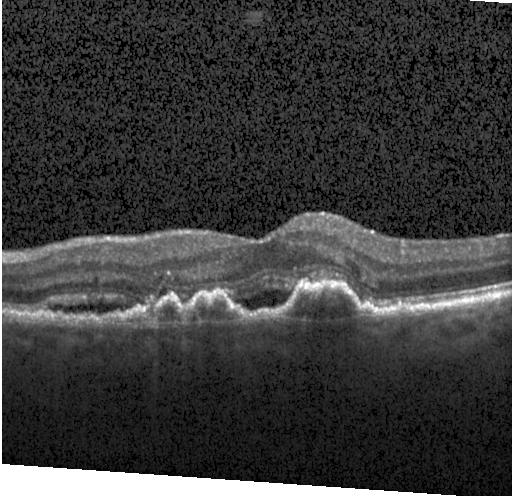

Spectral-domain optical coherence tomography · centered on the fovea · acquired on a Heidelberg Spectralis · optical coherence tomography B-scan — Dx: choroidal neovascularization.